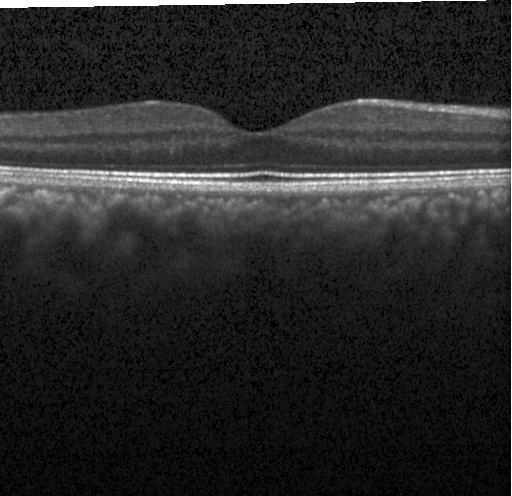
Through the macula. OCT line scan.
The scan shows no choroidal neovascularization, no diabetic macular edema, and no drusen.